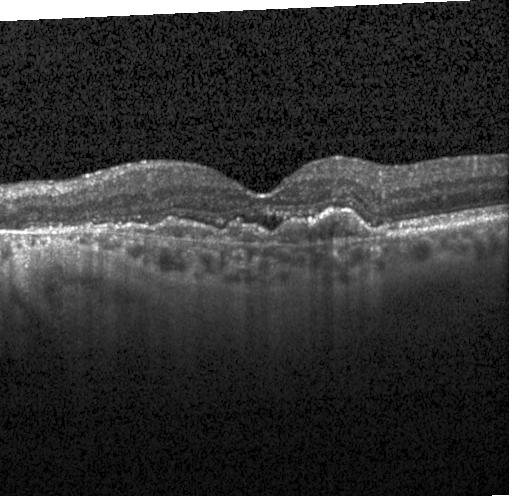

Finding: choroidal neovascularization.